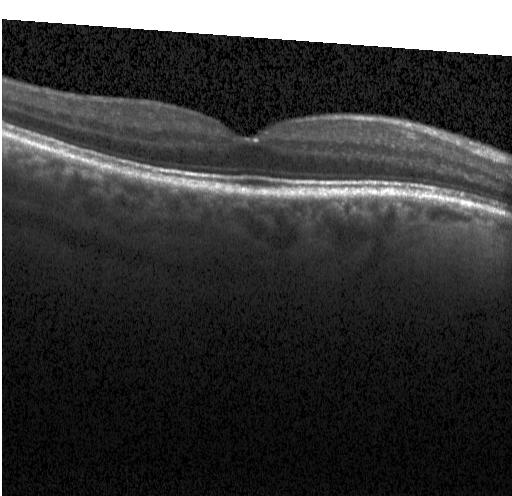 Spectral-domain optical coherence tomography · through the macula · OCT B-scan · Heidelberg Spectralis OCT system — No evidence of choroidal neovascularization, diabetic macular edema, or drusen.